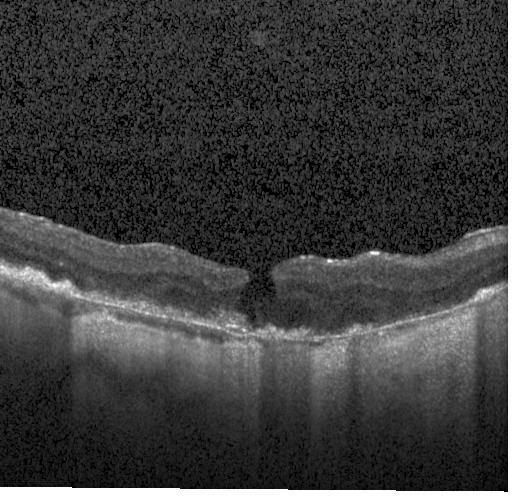
The scan shows choroidal neovascularization (CNV).